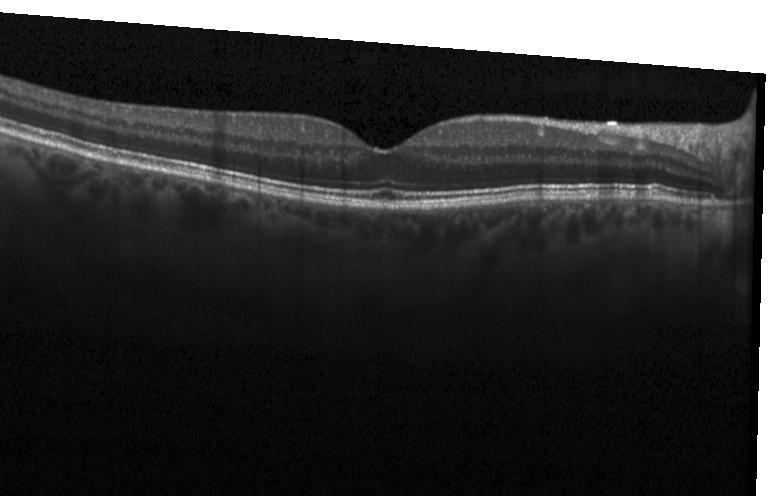

Retinal OCT B-scan — This B-scan demonstrates no evidence of choroidal neovascularization, diabetic macular edema, or drusen.